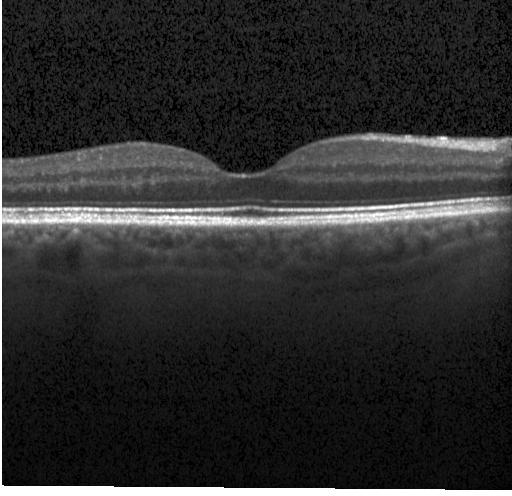 Acquired on a Heidelberg Spectralis · spectral-domain optical coherence tomography · optical coherence tomography scan. Impression: no CNV, no DME, and no drusen.